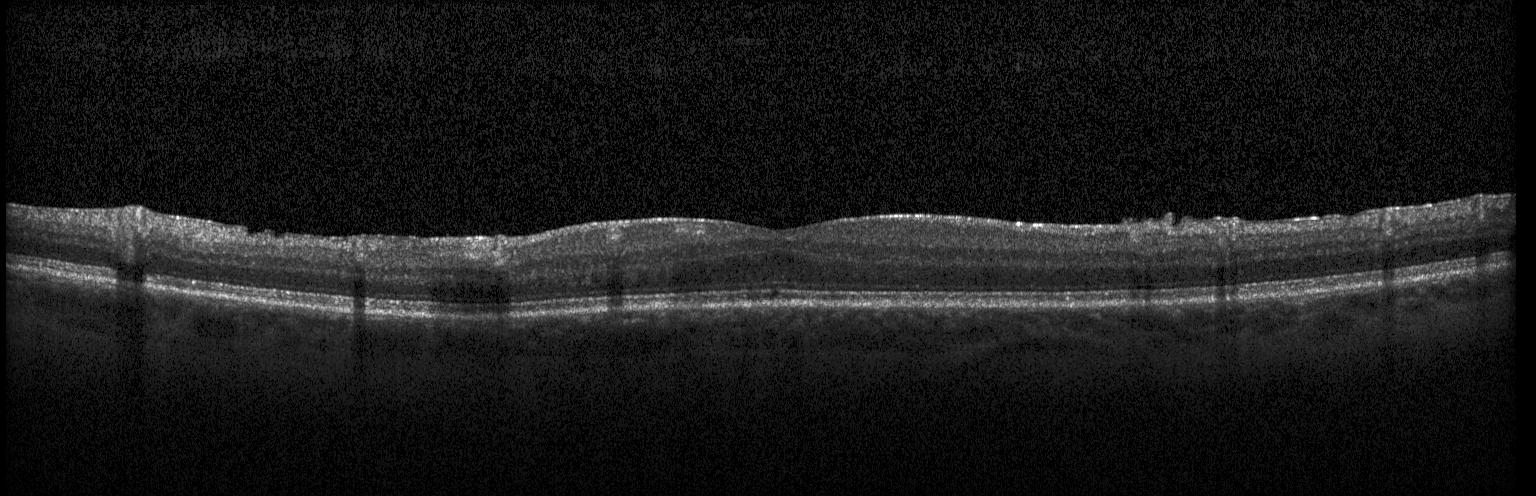

OCT B-scan showing no choroidal neovascularization, no diabetic macular edema, and no drusen.